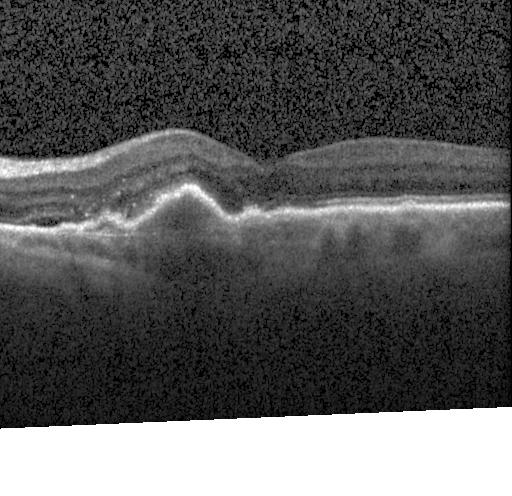 Optical coherence tomography B-scan, through the macula — Finding: choroidal neovascularization (CNV).